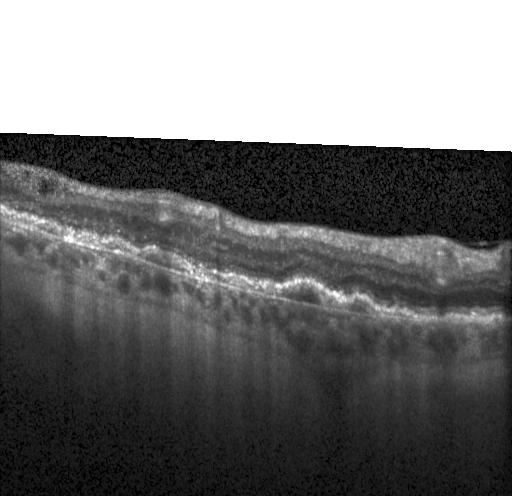
Optical coherence tomography scan, fovea-centered
A choroidal neovascular membrane.